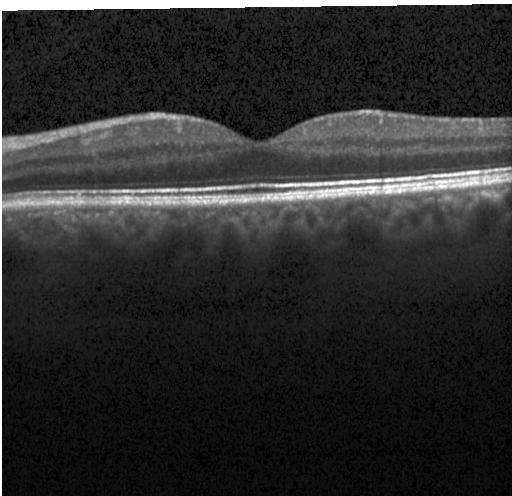

OCT line scan, fovea-centered.
OCT finding: no CNV, no DME, and no drusen.